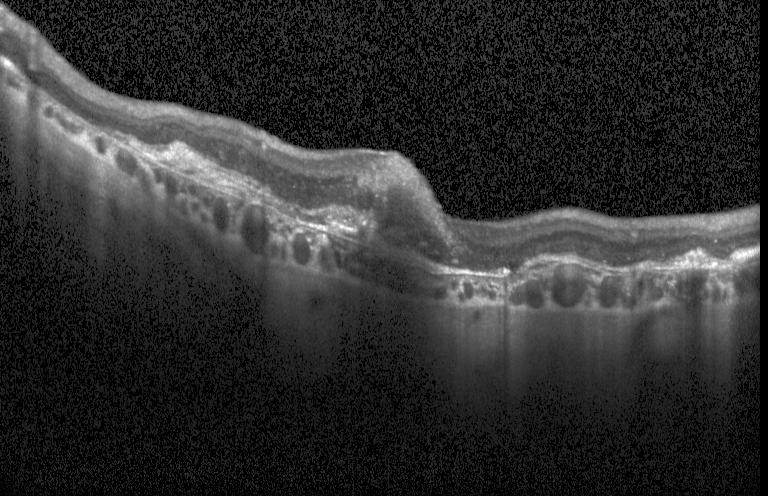 OCT B-scan. The scan shows choroidal neovascularization.